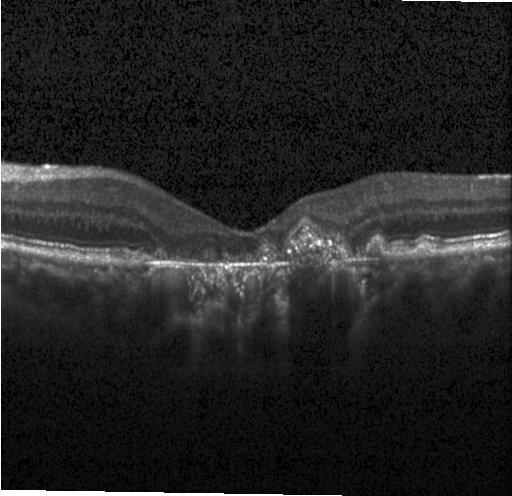

Retinal OCT cross-section.
Diagnosis: choroidal neovascularization.